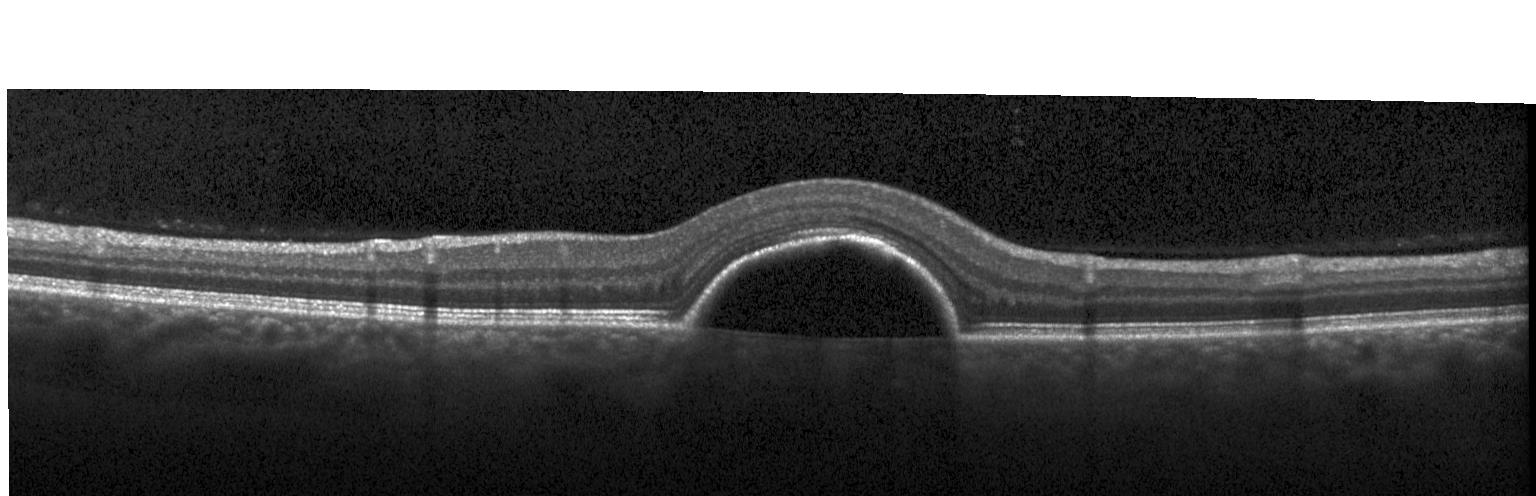
Spectral-domain OCT · OCT B-scan · instrument: Heidelberg Spectralis
Assessment: a choroidal neovascular membrane.